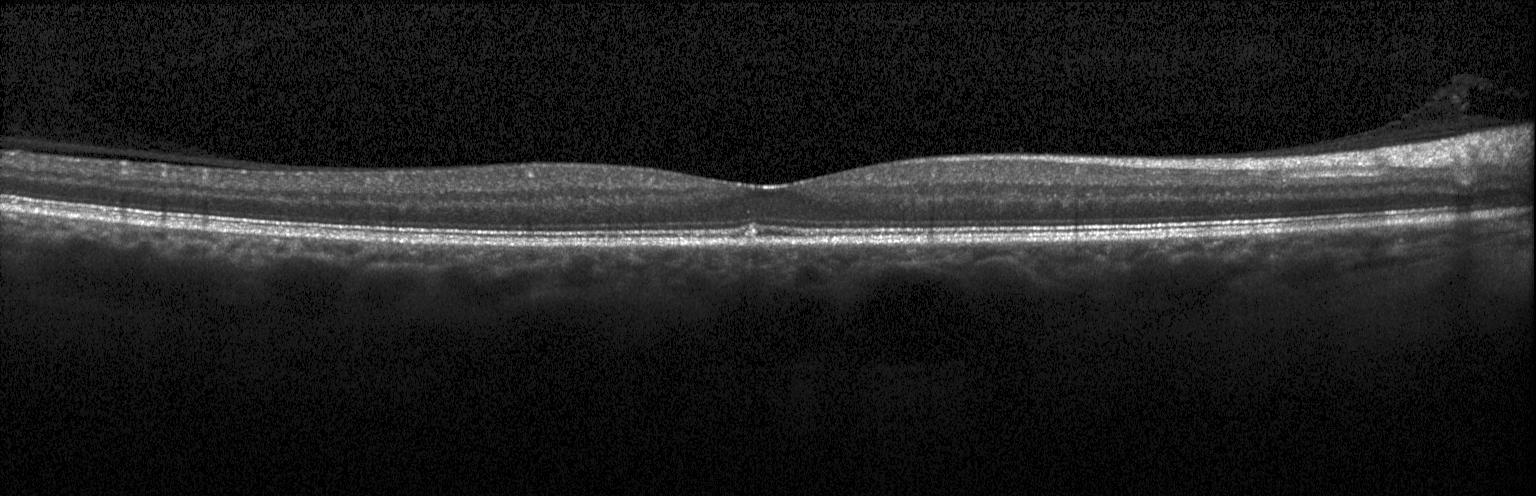

Retinal OCT B-scan.
Finding: drusen.